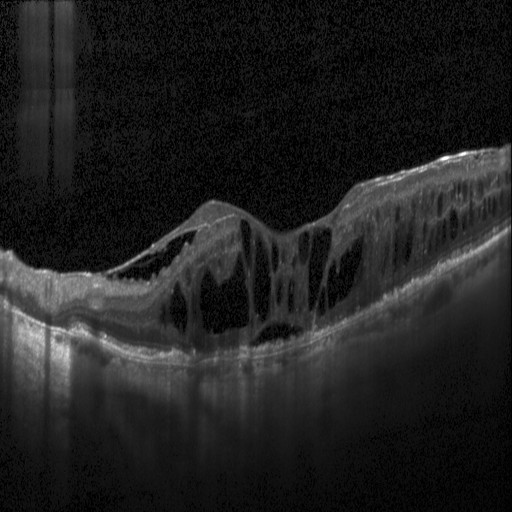

Retinal OCT cross-section. Spectral-domain OCT.
This B-scan demonstrates diabetic macular edema.